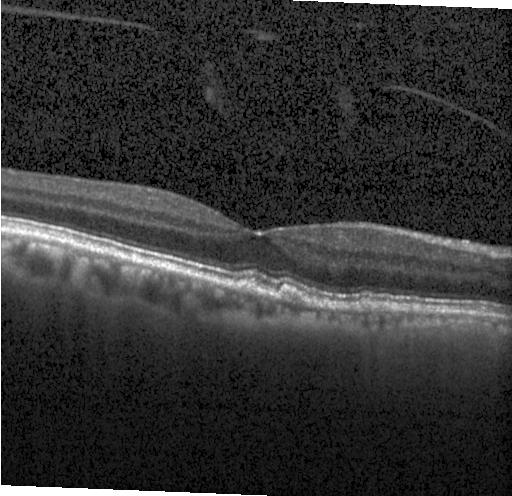 Heidelberg Spectralis OCT system · retinal OCT cross-section · macular scan · spectral-domain OCT — Macular OCT: sub-RPE drusenoid deposits.